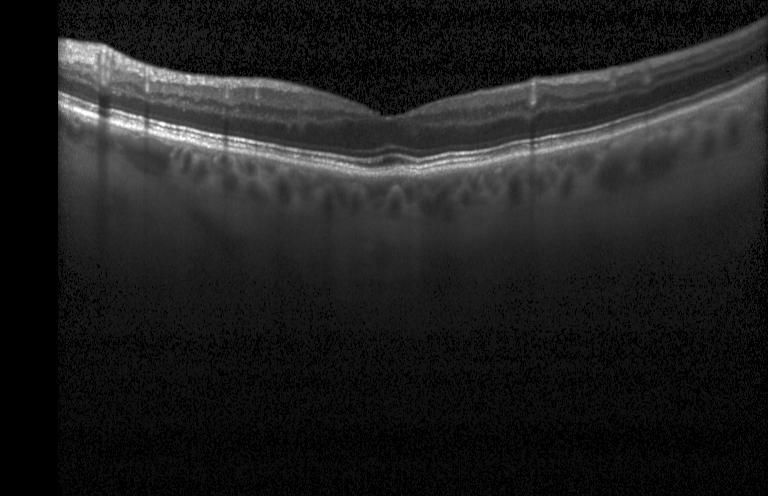 Spectral-domain OCT · Heidelberg Spectralis OCT system · fovea-centered · OCT B-scan
OCT finding: neither choroidal neovascularization, diabetic macular edema, nor drusen.